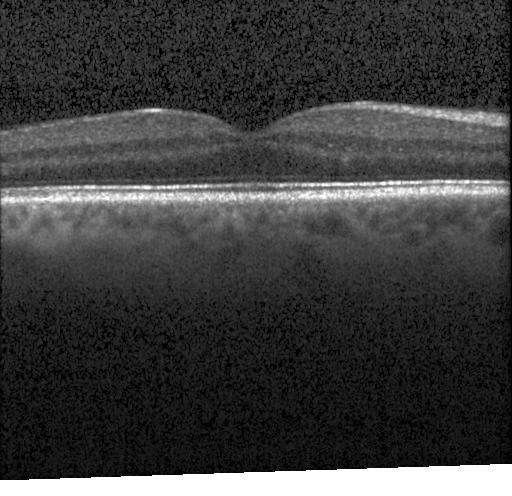

Heidelberg Spectralis · centered on the fovea · retinal OCT B-scan · SD-OCT. Diagnosis: neither choroidal neovascularization, diabetic macular edema, nor drusen.